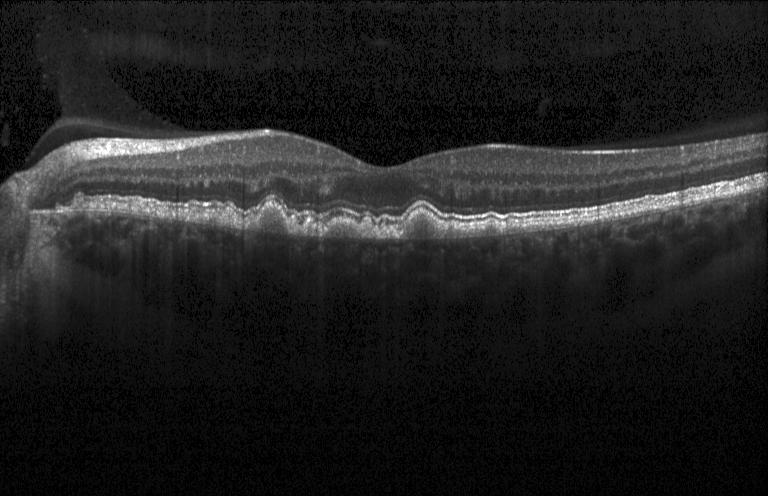
Retinal OCT B-scan; SD-OCT.
Impression: drusen.